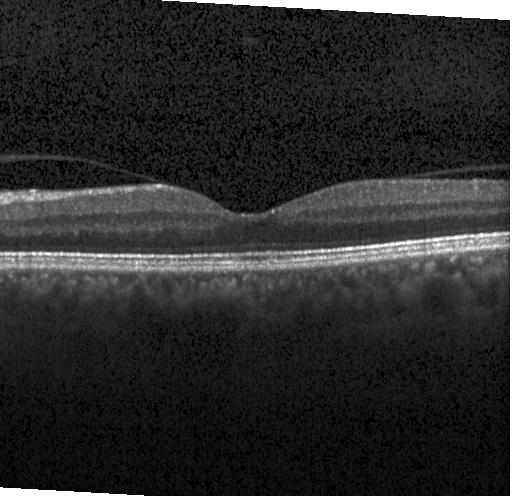

Finding: no choroidal neovascularization, no diabetic macular edema, and no drusen.